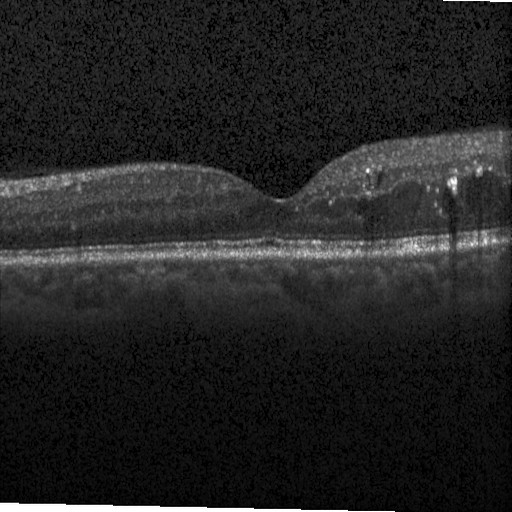 Retinal OCT B-scan · Heidelberg Spectralis · SD-OCT · centered on the fovea.
Macular OCT: DME.